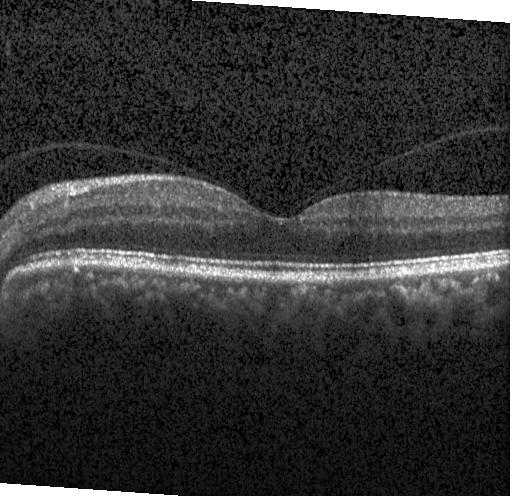
Diagnosis: no choroidal neovascularization, diabetic macular edema, or drusen.